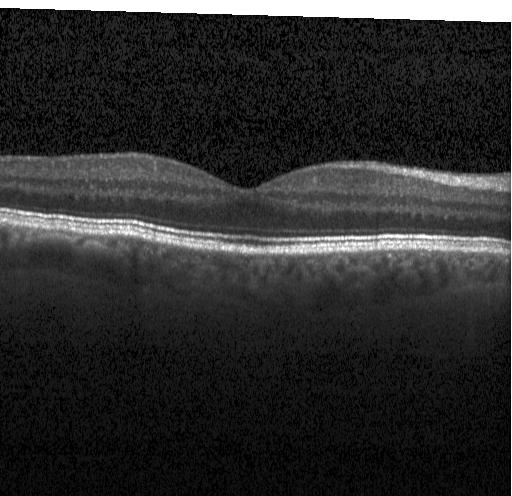 Optical coherence tomography scan.
Diagnosis: no evidence of choroidal neovascularization, diabetic macular edema, or drusen.